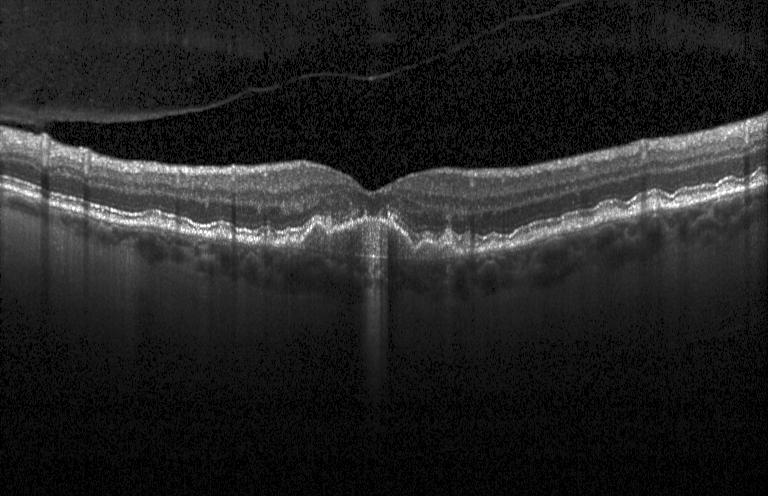

Finding: a choroidal neovascular membrane.